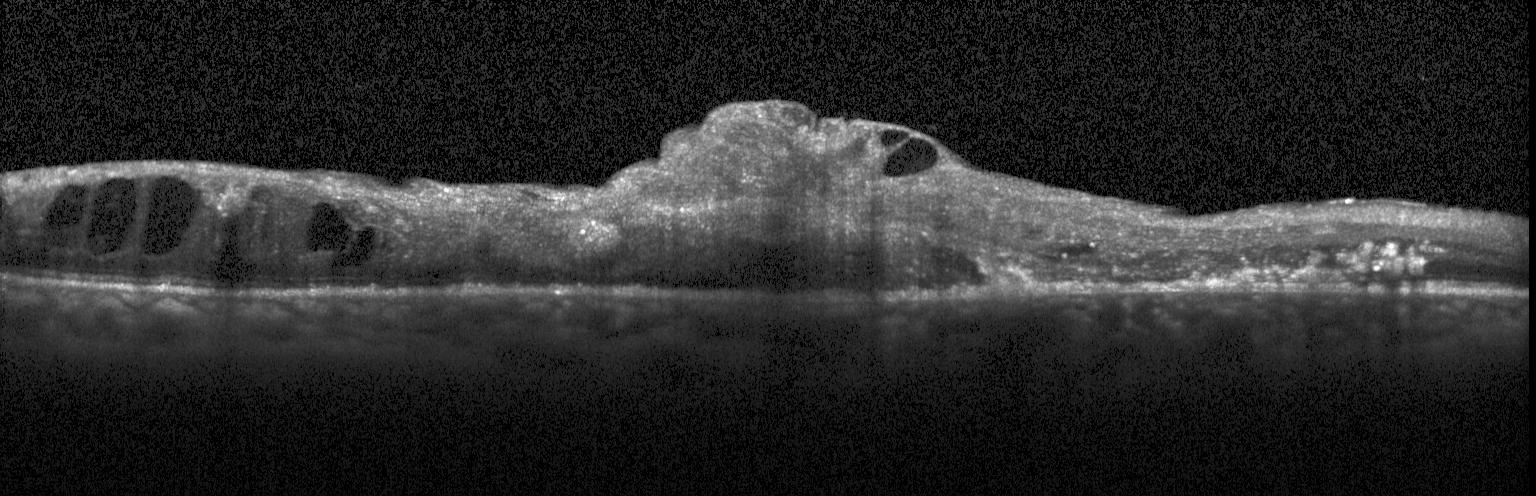 Spectral-domain OCT · horizontal scan through the fovea · retinal OCT cross-section · Heidelberg Spectralis — Choroidal neovascularization.